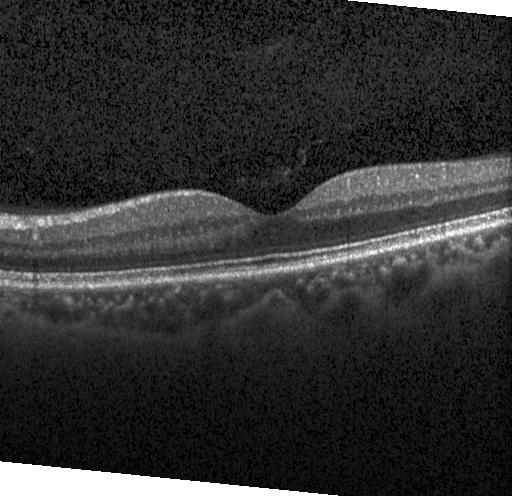 Spectral-domain OCT. Horizontal scan through the fovea. Retinal OCT cross-section. Neither CNV, DME, nor drusen.